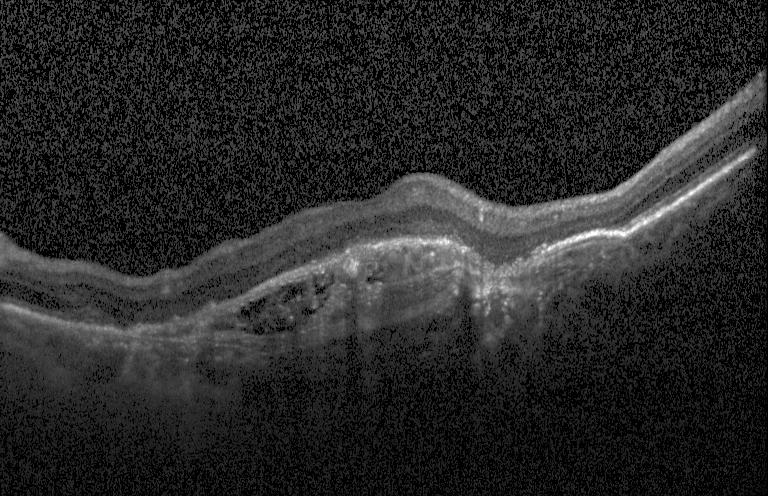
Through the macula, Heidelberg Spectralis, retinal OCT B-scan
Assessment: a choroidal neovascular membrane.